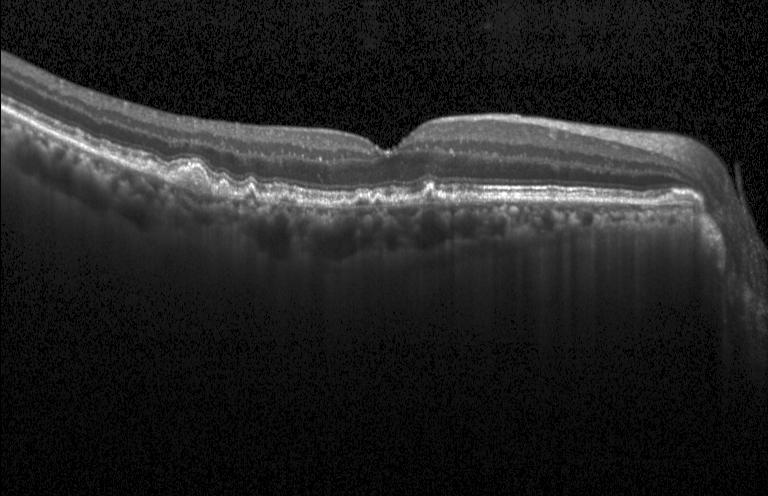 Retinal OCT cross-section — Dx: multiple drusen.